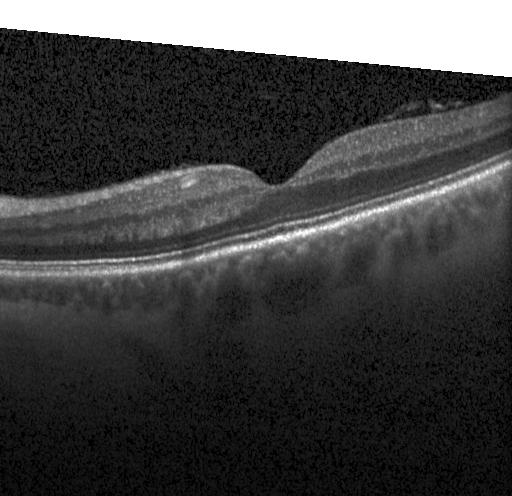
Impression: neither choroidal neovascularization, diabetic macular edema, nor drusen.